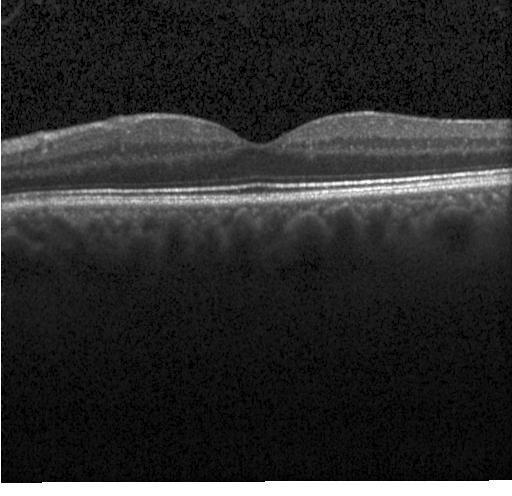
Retinal OCT B-scan · fovea-centered
Diagnosis: no CNV, DME, or drusen.